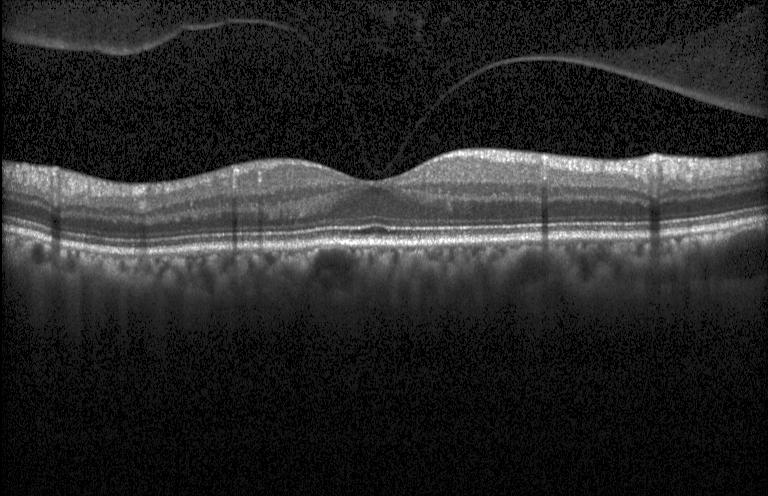
The scan shows no choroidal neovascularization, no diabetic macular edema, and no drusen.